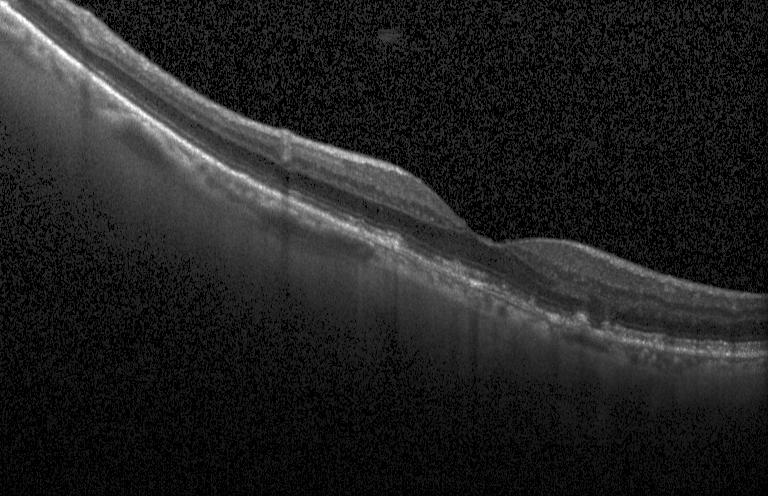
Spectral-domain OCT B-scan: sub-RPE drusenoid deposits.